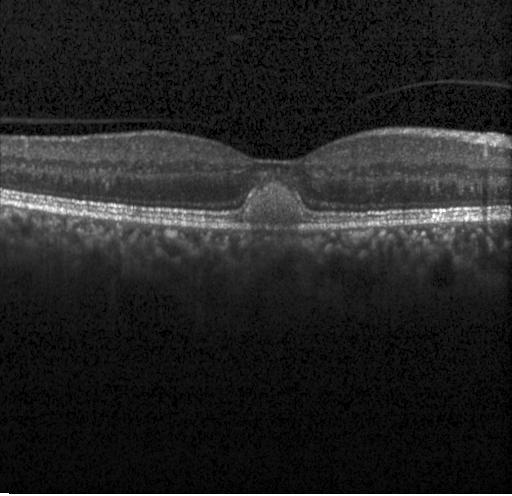
Spectral-domain OCT B-scan: a choroidal neovascular membrane.